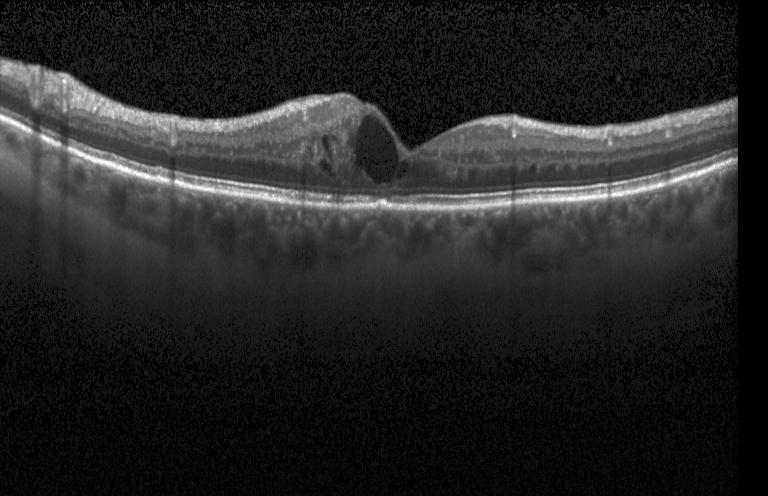 Heidelberg Spectralis · optical coherence tomography scan · SD-OCT
Diabetic macular edema (DME).